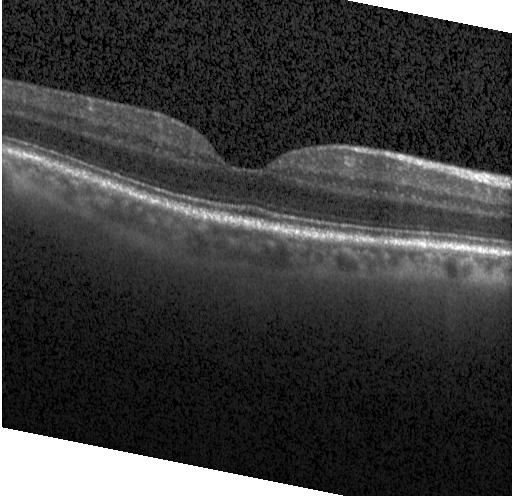
Spectral-domain optical coherence tomography. Optical coherence tomography scan. No evidence of choroidal neovascularization, diabetic macular edema, or drusen.